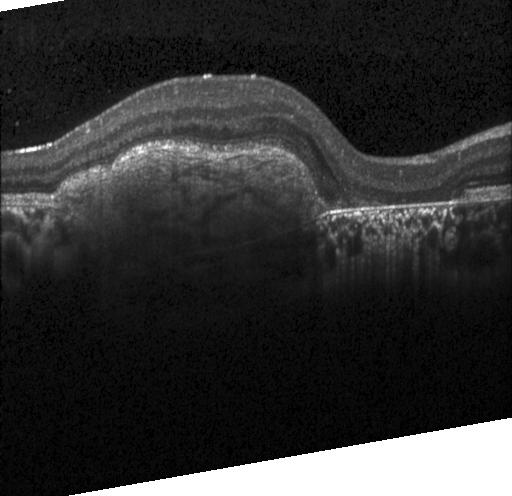
A choroidal neovascular membrane.